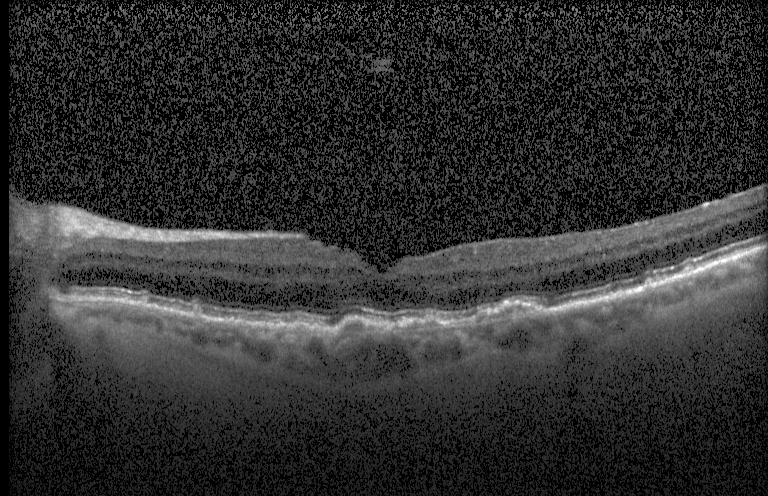

Centered on the fovea; OCT line scan
This B-scan demonstrates drusen.